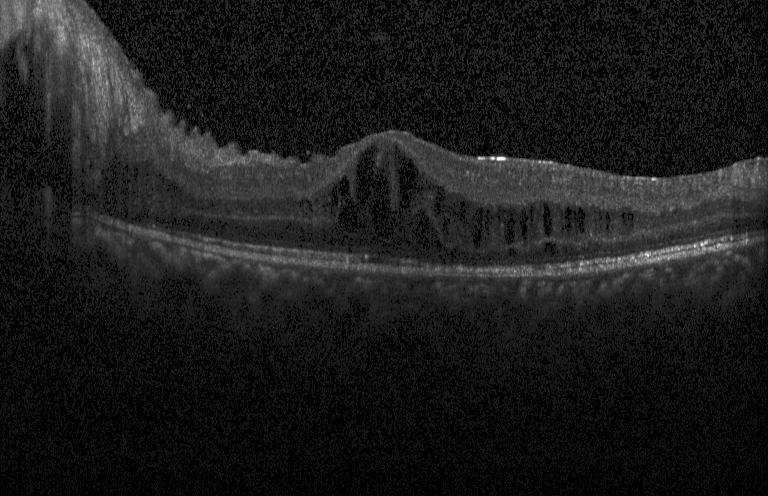
Heidelberg Spectralis OCT system, optical coherence tomography scan, spectral-domain optical coherence tomography, horizontal scan through the fovea
Impression: diabetic macular edema.